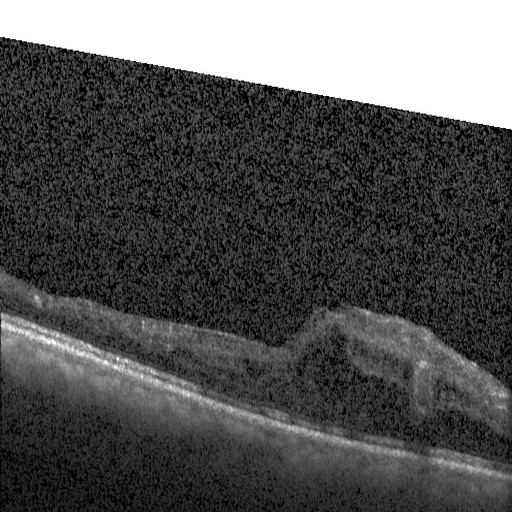 Optical coherence tomography scan
Assessment: diabetic macular edema.